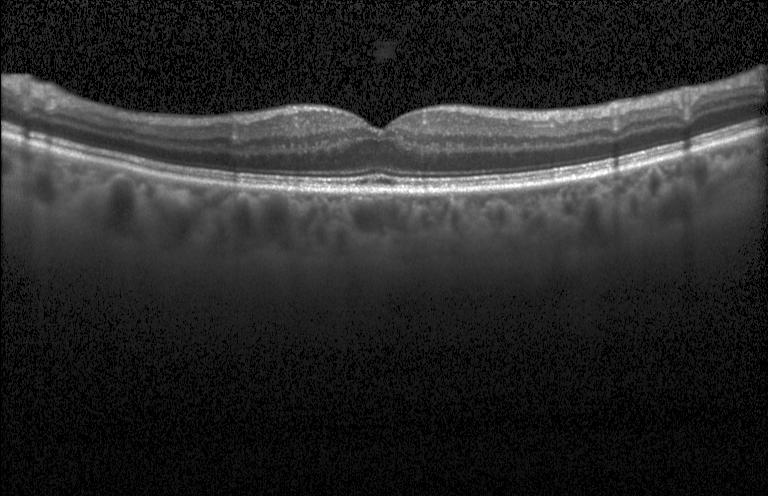
Heidelberg Spectralis OCT system; fovea-centered; SD-OCT; retinal OCT B-scan. Diagnosis: no choroidal neovascularization, no diabetic macular edema, and no drusen.